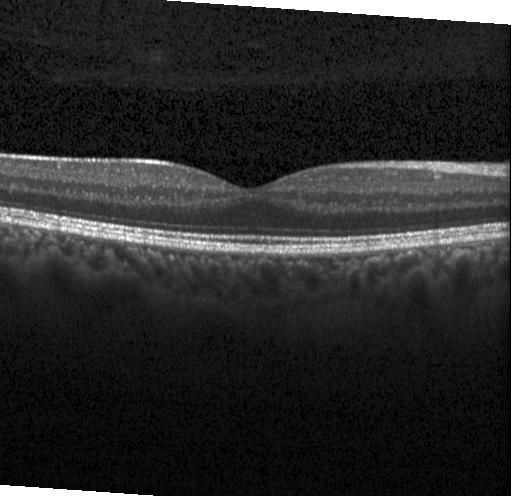

Spectral-domain optical coherence tomography; OCT B-scan — Assessment: no CNV, DME, or drusen.